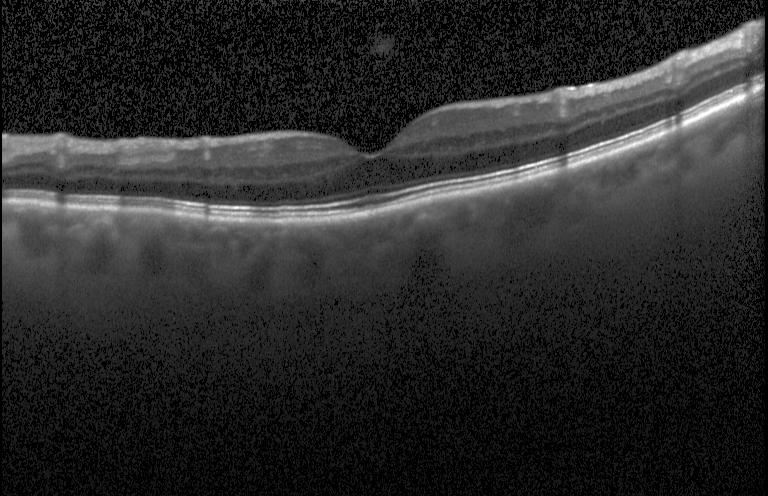 Spectral-domain optical coherence tomography, Heidelberg Spectralis OCT system, retinal OCT cross-section, centered on the fovea — Diagnosis: no evidence of choroidal neovascularization, diabetic macular edema, or drusen.